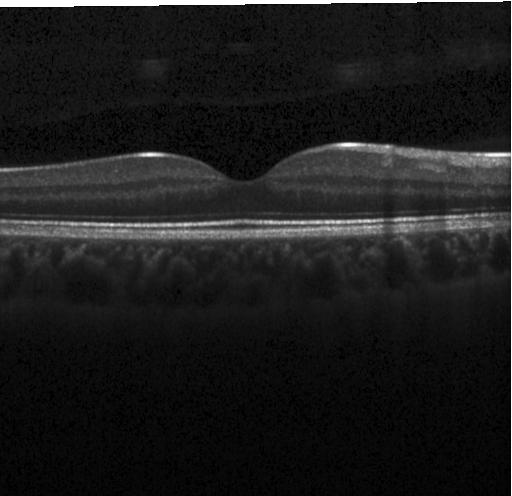
Dx: neither choroidal neovascularization, diabetic macular edema, nor drusen.